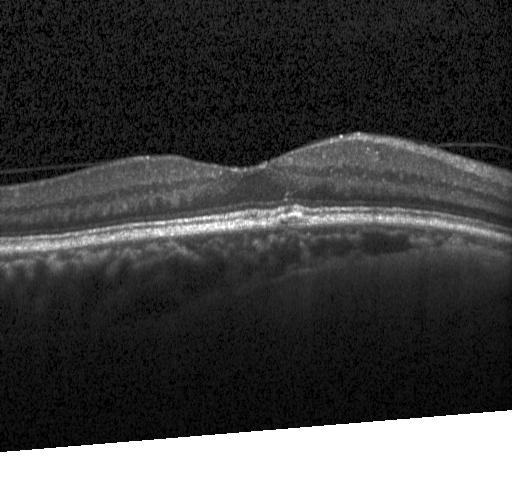

Retinal OCT cross-section · SD-OCT
Finding: multiple drusen.